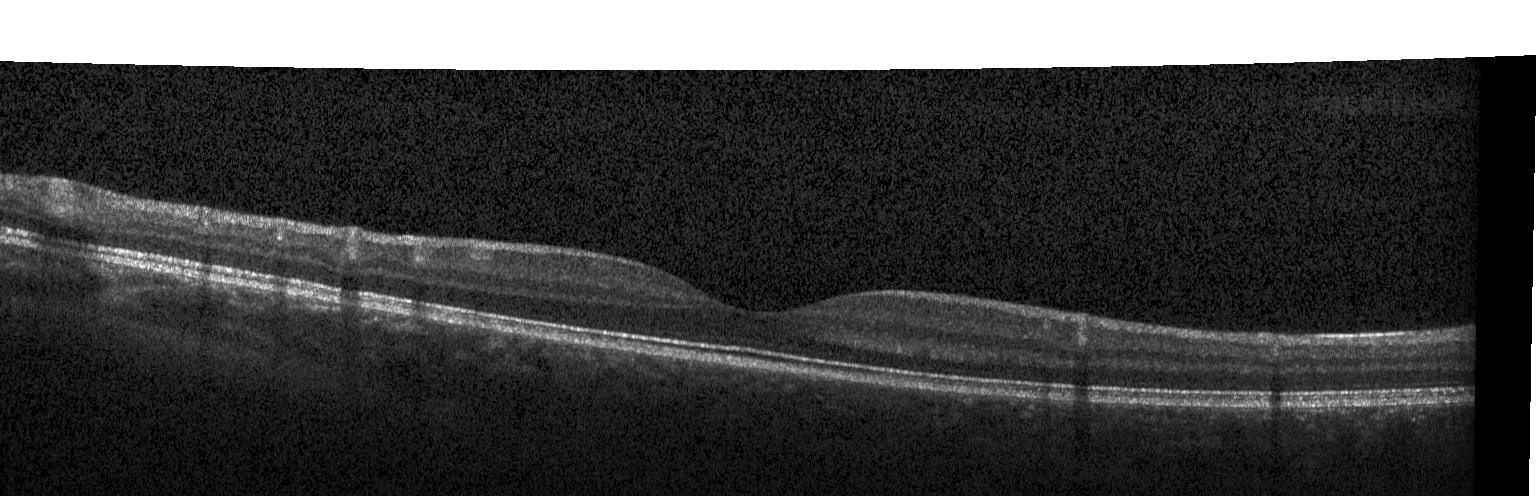
OCT line scan; fovea-centered.
Macular OCT: no evidence of CNV, DME, or drusen.